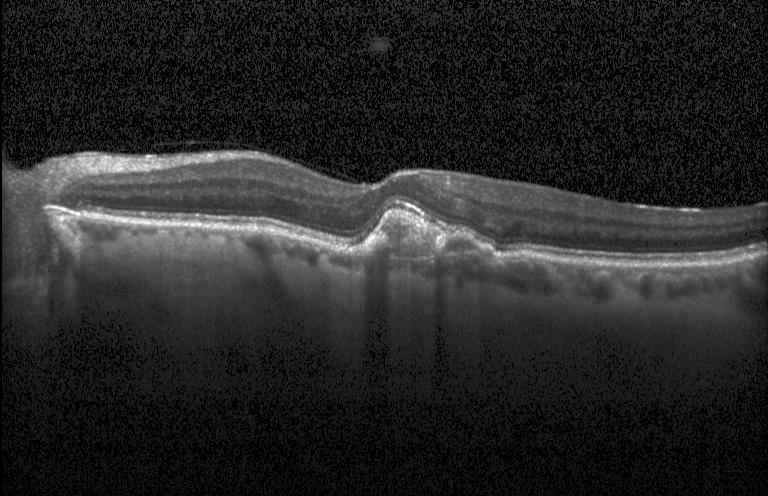 OCT B-scan showing a choroidal neovascular membrane.